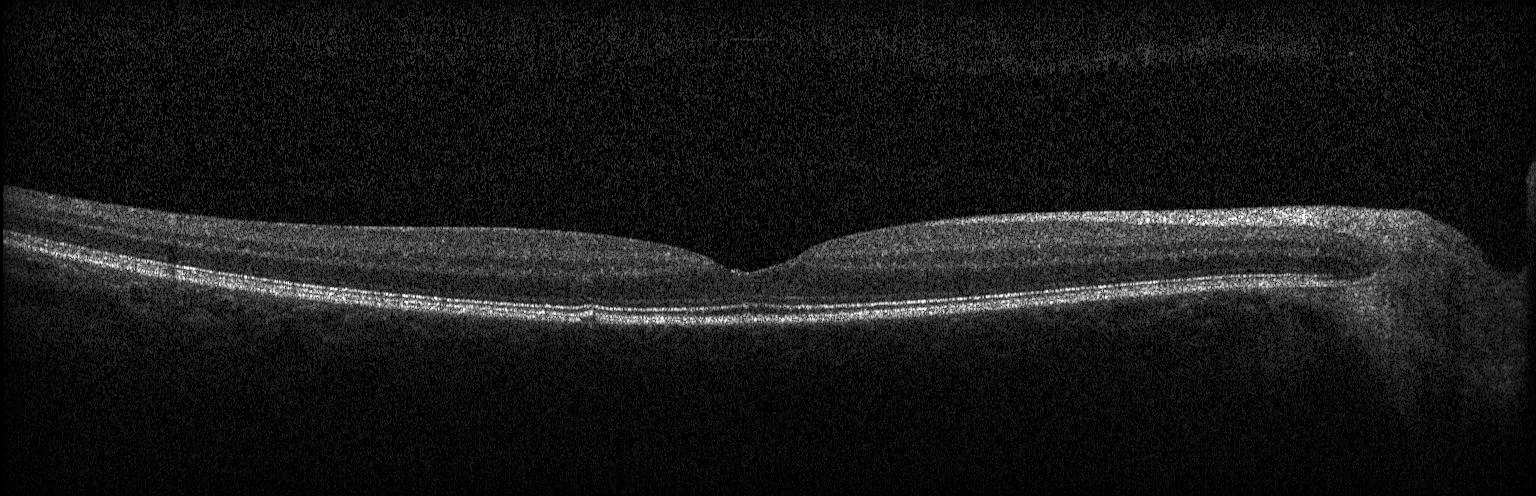

OCT finding: no CNV, DME, or drusen.